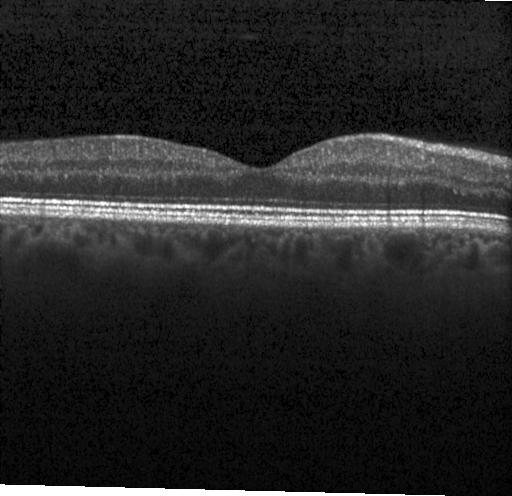

Diagnosis: neither choroidal neovascularization, diabetic macular edema, nor drusen.